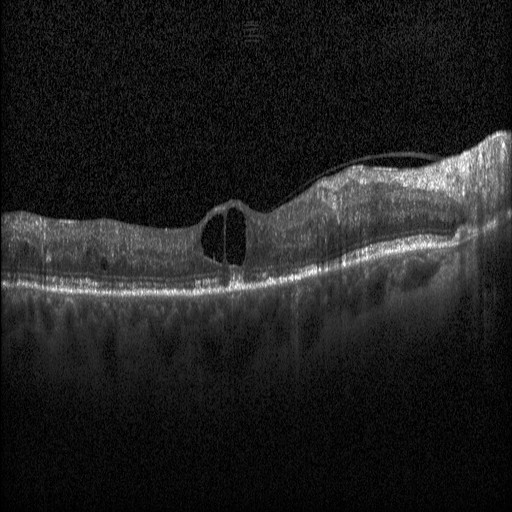 OCT finding: DME.